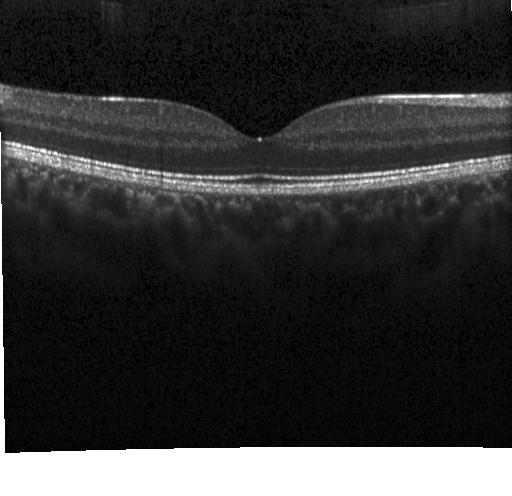 Retinal OCT cross-section — Impression: neither choroidal neovascularization, diabetic macular edema, nor drusen.